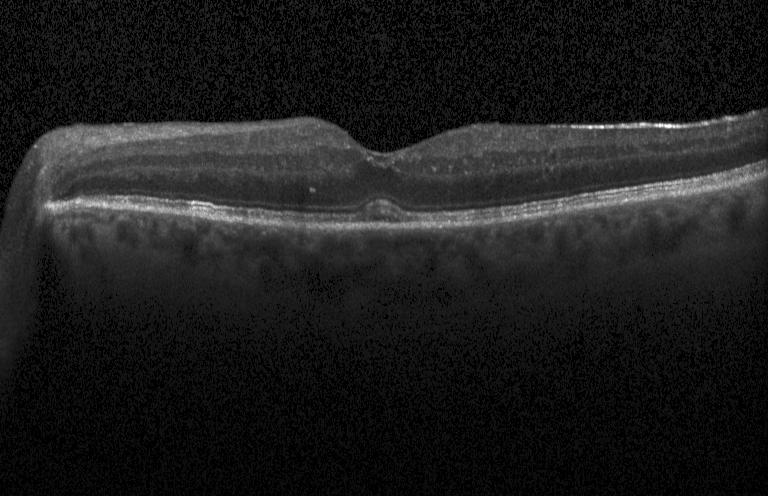
OCT B-scan
Diagnosis: DME.